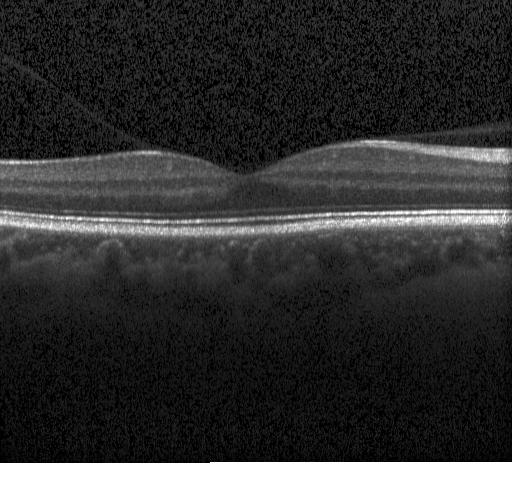

OCT B-scan; instrument: Heidelberg Spectralis; through the macula. Finding: no evidence of choroidal neovascularization, diabetic macular edema, or drusen.